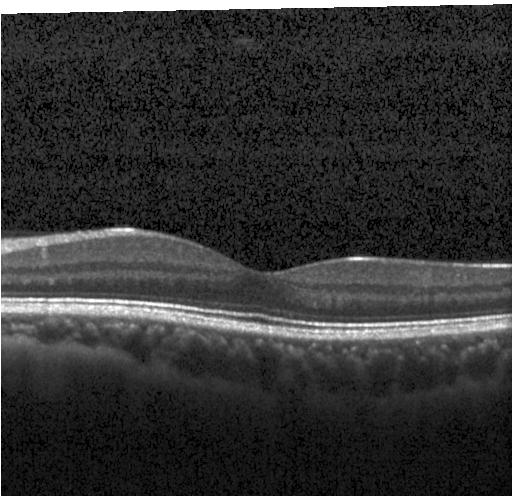

Optical coherence tomography B-scan. Heidelberg Spectralis OCT system. Spectral-domain optical coherence tomography. Macular scan — No evidence of CNV, DME, or drusen.